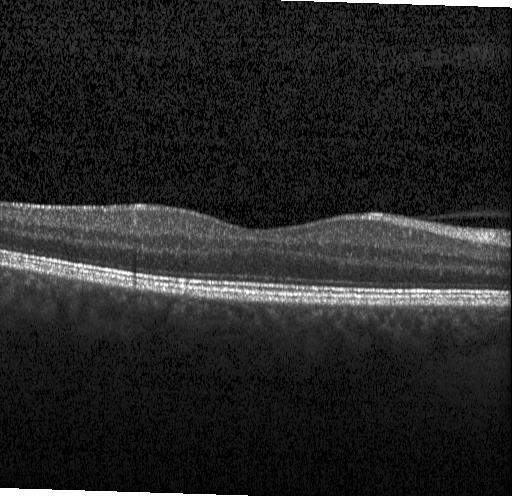
Diagnosis: no choroidal neovascularization, no diabetic macular edema, and no drusen.